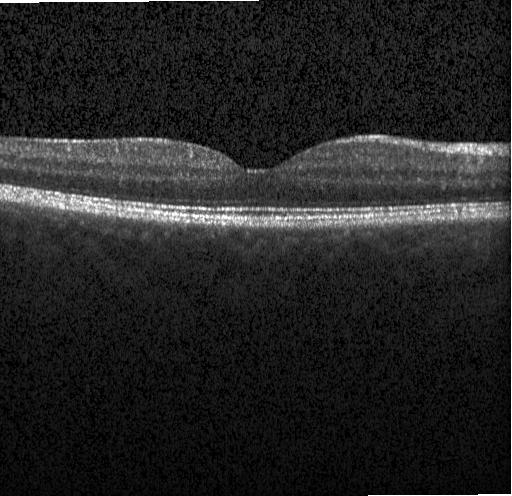
Dx: no choroidal neovascularization, diabetic macular edema, or drusen.